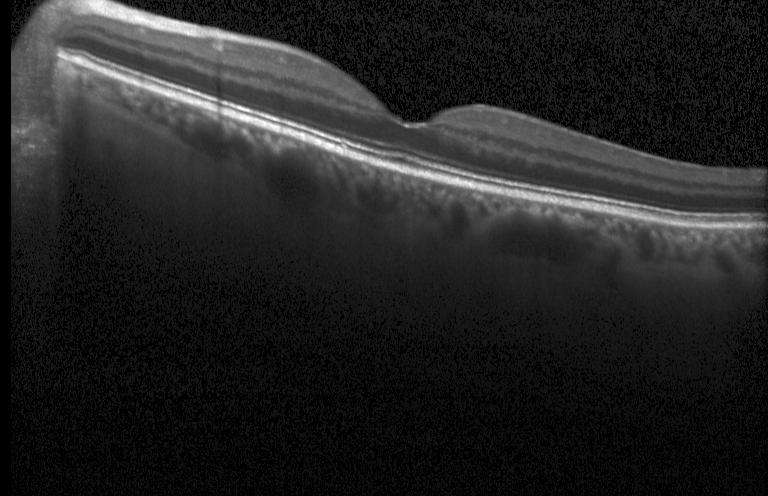

OCT finding: no evidence of choroidal neovascularization, diabetic macular edema, or drusen.